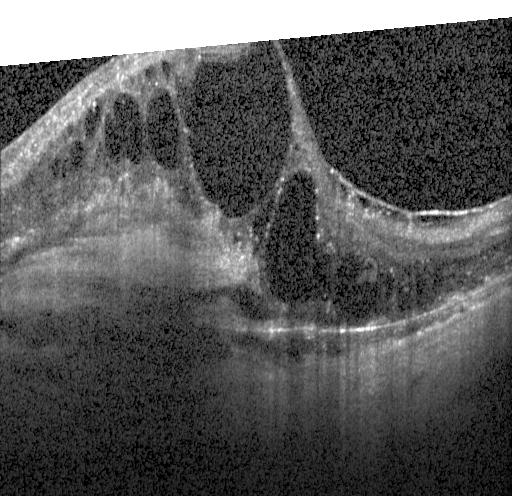 Dx: CNV.